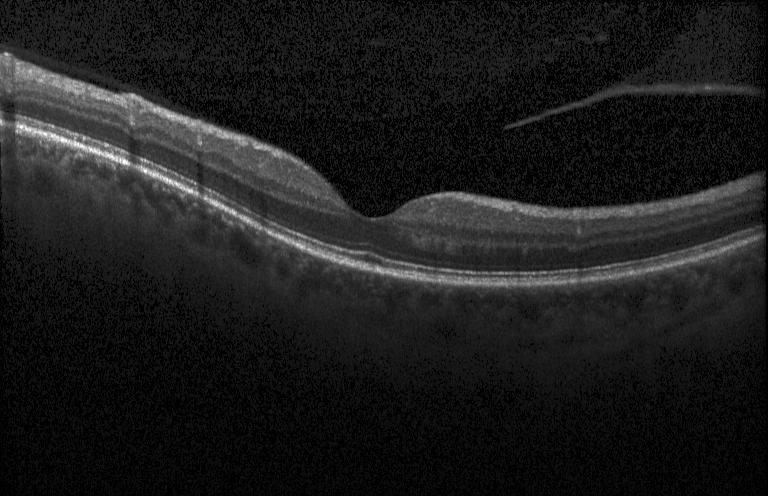
Retinal OCT cross-section. Macular scan. Heidelberg Spectralis OCT system. Spectral-domain optical coherence tomography
The scan shows no evidence of choroidal neovascularization, diabetic macular edema, or drusen.